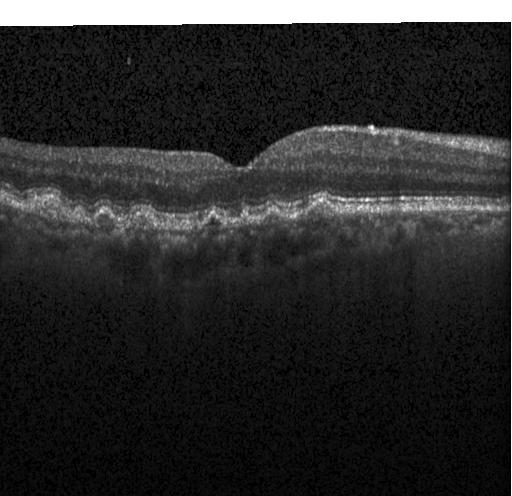
Instrument: Heidelberg Spectralis, through the macula, OCT B-scan, SD-OCT.
The scan shows sub-RPE drusenoid deposits.